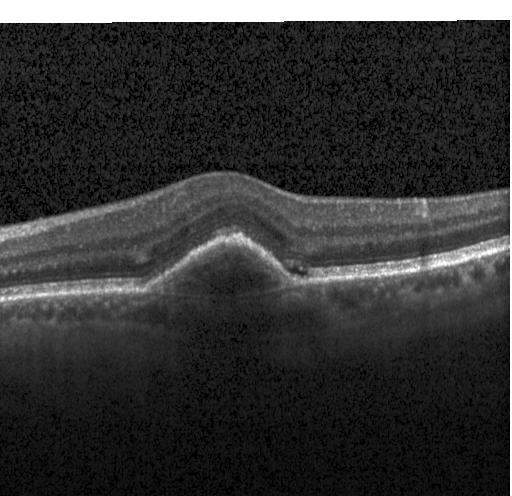

Instrument: Heidelberg Spectralis, SD-OCT, OCT B-scan
Impression: choroidal neovascularization (CNV).